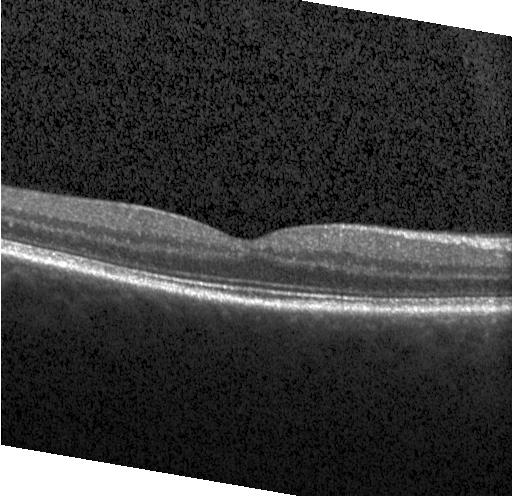 OCT line scan. Through the macula
Finding: no CNV, no DME, and no drusen.